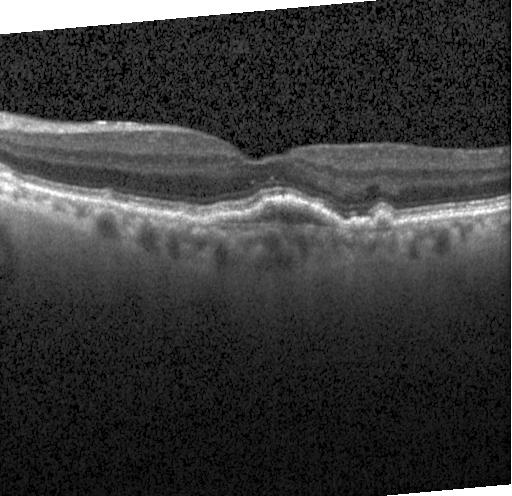

Diagnosis: choroidal neovascularization (CNV).